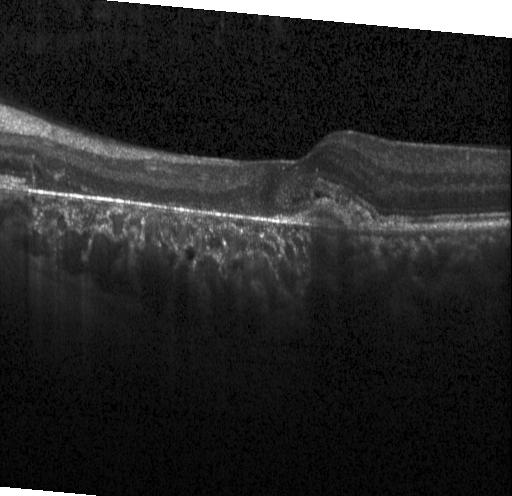

Macular OCT: a choroidal neovascular membrane.